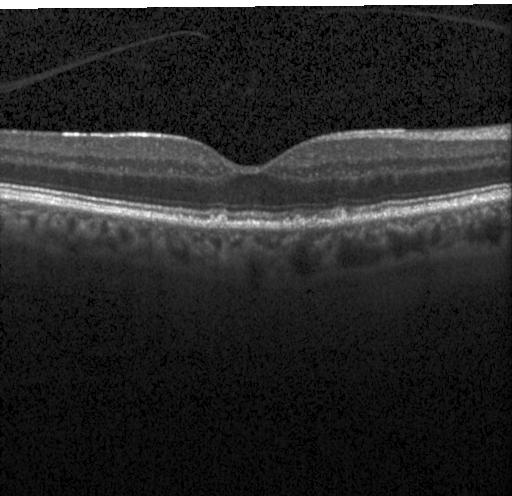
OCT line scan. Macular scan
Multiple drusen.